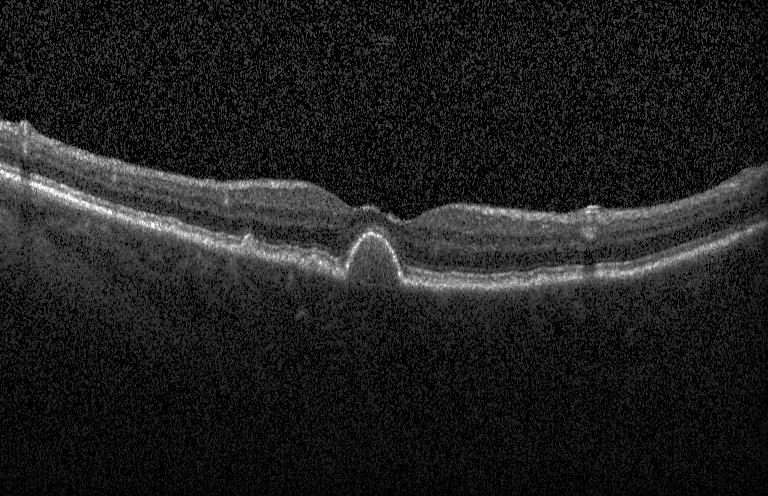 OCT scan showing drusen.